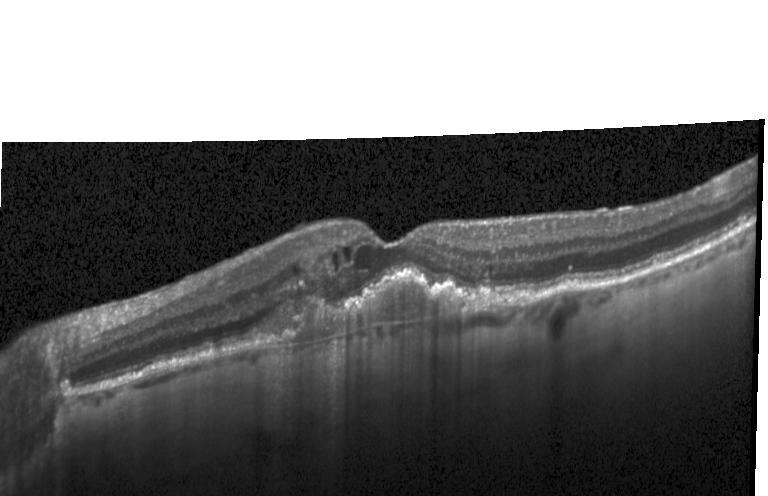

Impression: choroidal neovascularization.